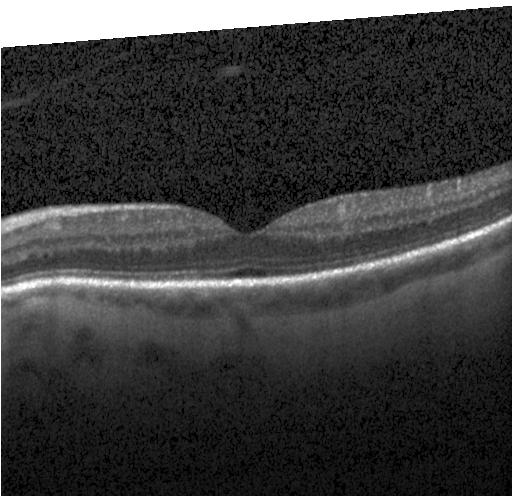 OCT scan showing no CNV, DME, or drusen.